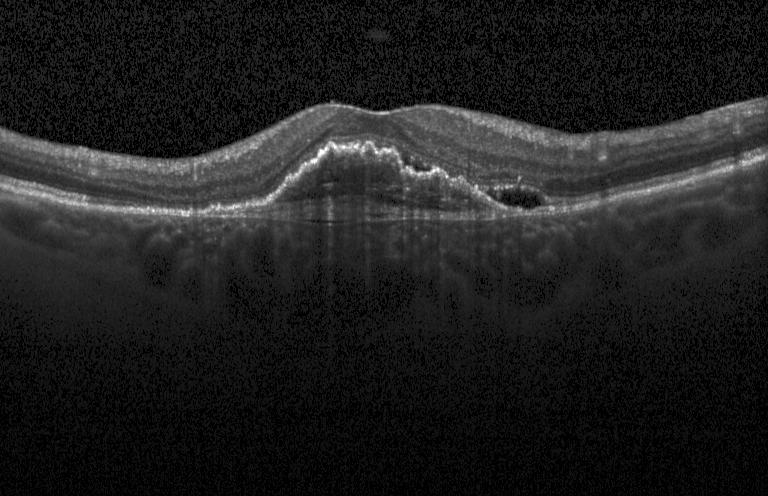 Horizontal scan through the fovea. Retinal OCT B-scan.
The scan shows CNV.